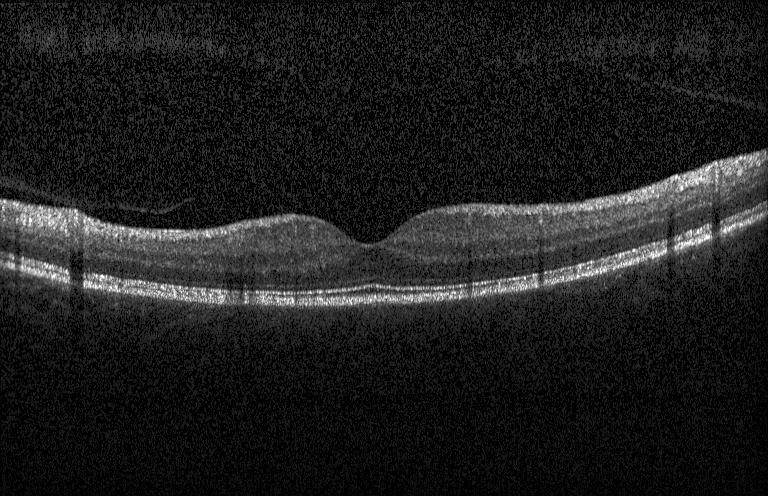 SD-OCT; OCT B-scan; instrument: Heidelberg Spectralis.
Finding: neither choroidal neovascularization, diabetic macular edema, nor drusen.